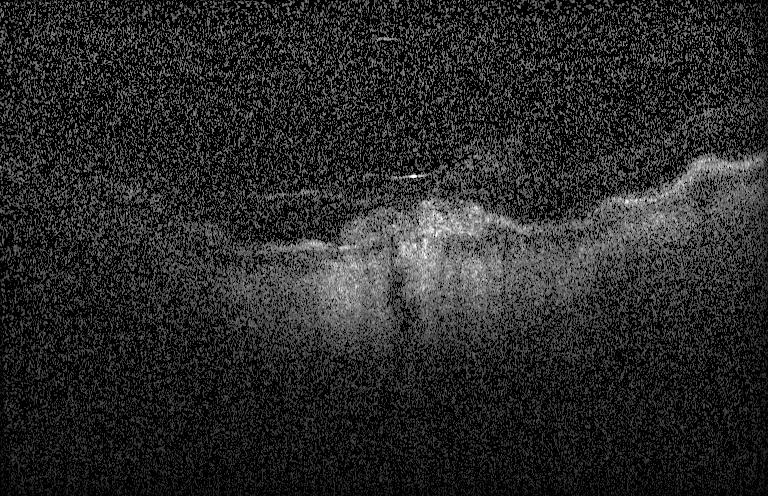
Through the macula, Heidelberg Spectralis, retinal OCT cross-section, spectral-domain OCT — Impression: CNV.